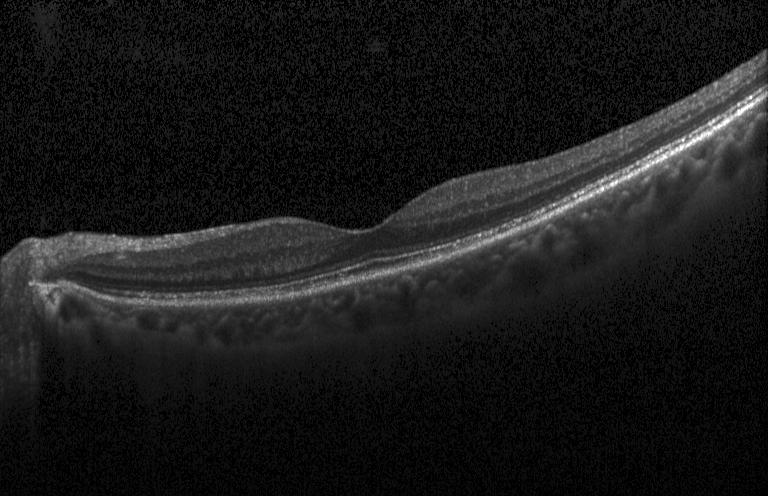

OCT B-scan showing neither choroidal neovascularization, diabetic macular edema, nor drusen.